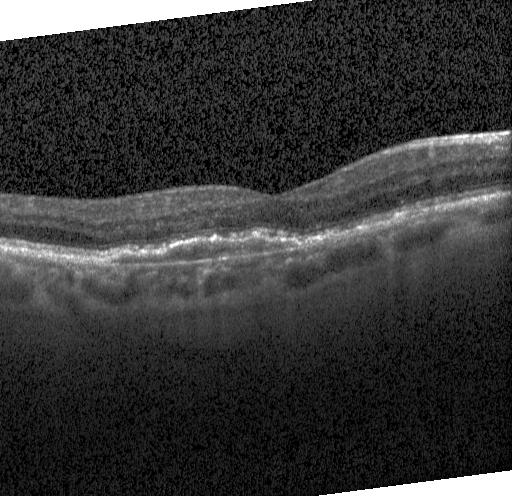
Acquired on a Heidelberg Spectralis. Optical coherence tomography scan. Dx: CNV.